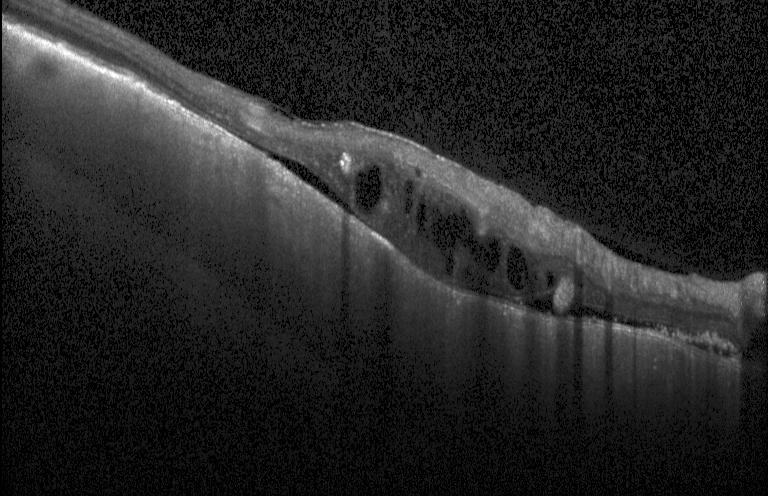
Optical coherence tomography scan.
Finding: choroidal neovascularization.